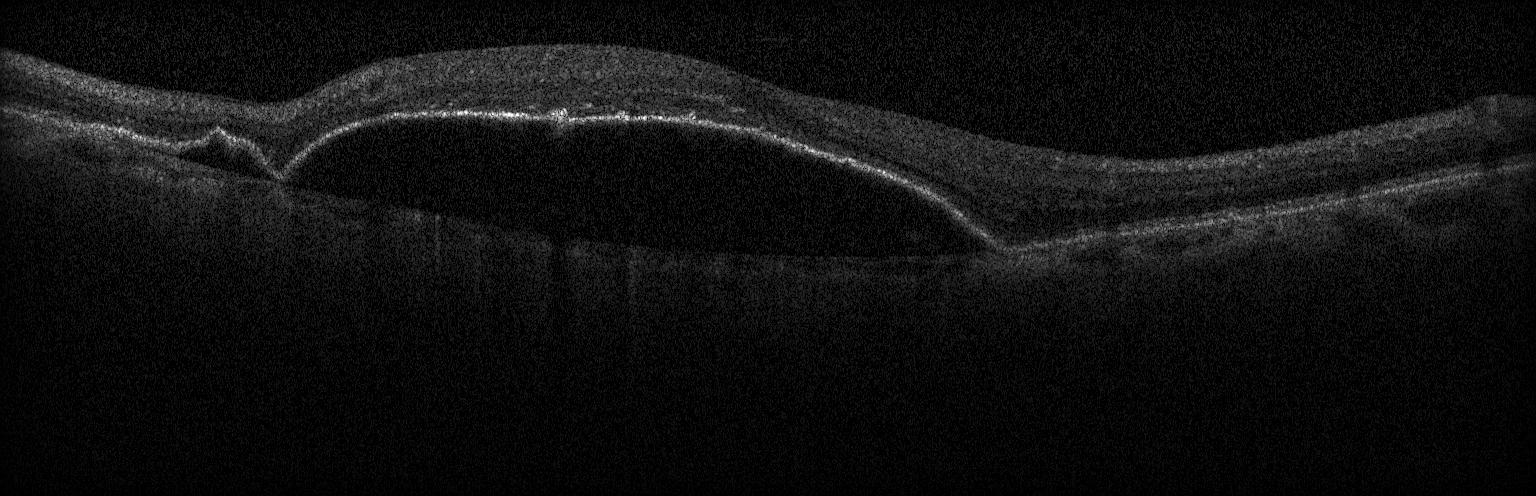

OCT B-scan
Assessment: CNV.